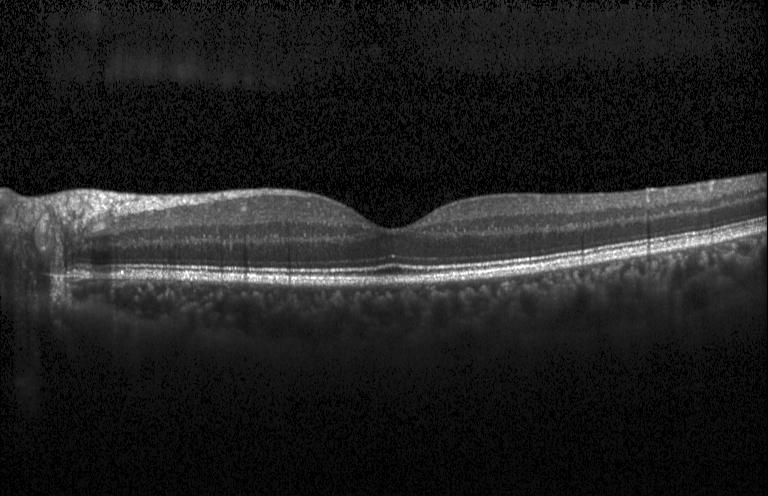

Macular scan; spectral-domain optical coherence tomography; acquired on a Heidelberg Spectralis; retinal OCT cross-section.
Assessment: no choroidal neovascularization, no diabetic macular edema, and no drusen.